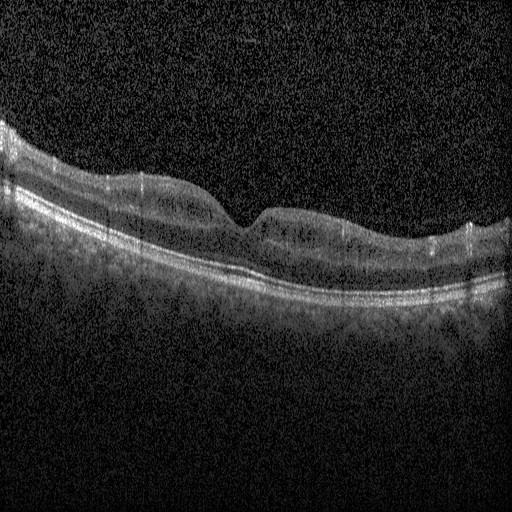
Macular OCT demonstrating DME.